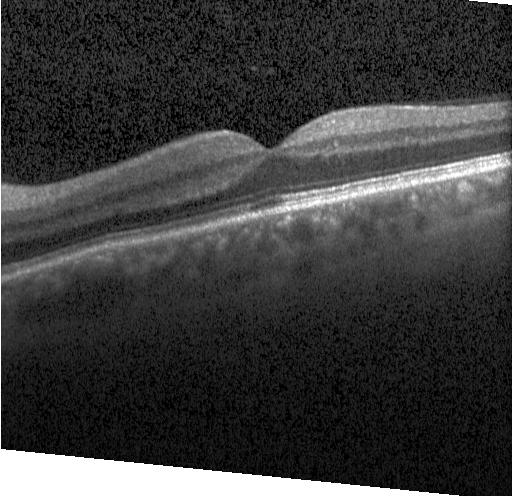 Retinal OCT cross-section; spectral-domain optical coherence tomography; Heidelberg Spectralis. The scan shows no choroidal neovascularization, no diabetic macular edema, and no drusen.